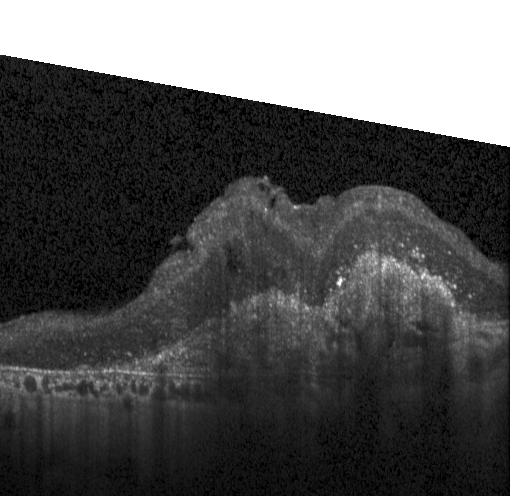 Heidelberg Spectralis. Retinal OCT B-scan. Spectral-domain OCT. Centered on the fovea. Assessment: a choroidal neovascular membrane.